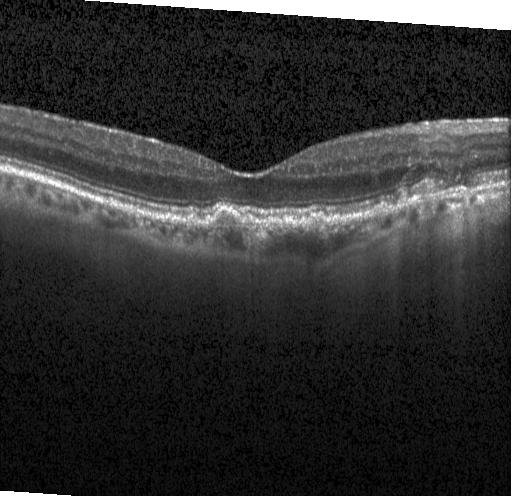

Impression: drusen.